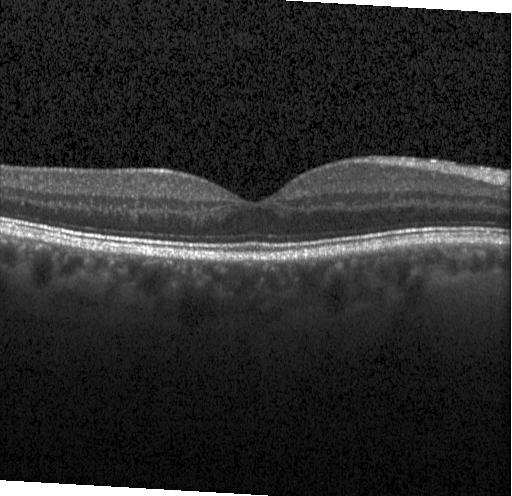
OCT B-scan. Macular OCT: no choroidal neovascularization, no diabetic macular edema, and no drusen.